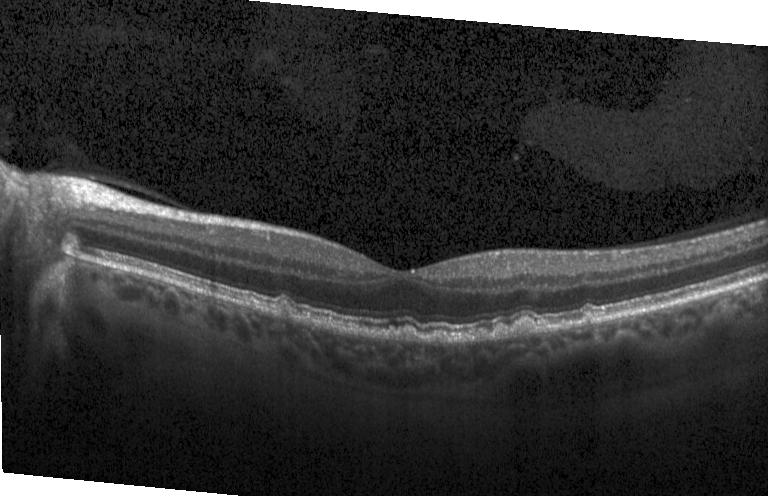

Fovea-centered · retinal OCT B-scan · Heidelberg Spectralis.
Finding: drusen.